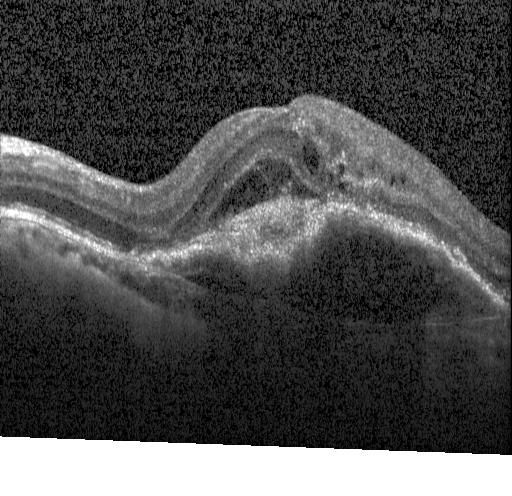
Retinal OCT cross-section. Spectral-domain OCT. Instrument: Heidelberg Spectralis — Impression: a choroidal neovascular membrane.